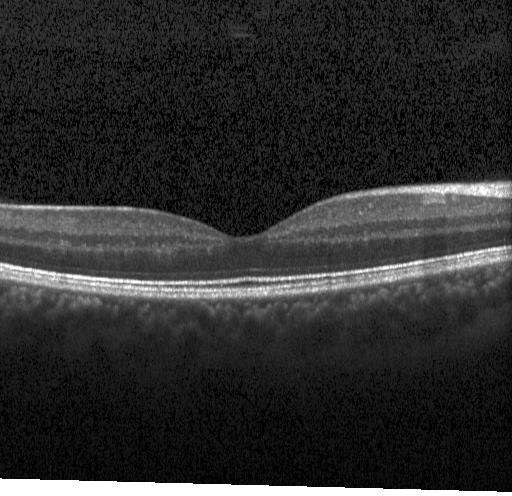
Instrument: Heidelberg Spectralis, SD-OCT, retinal OCT B-scan
Diagnosis: no evidence of choroidal neovascularization, diabetic macular edema, or drusen.